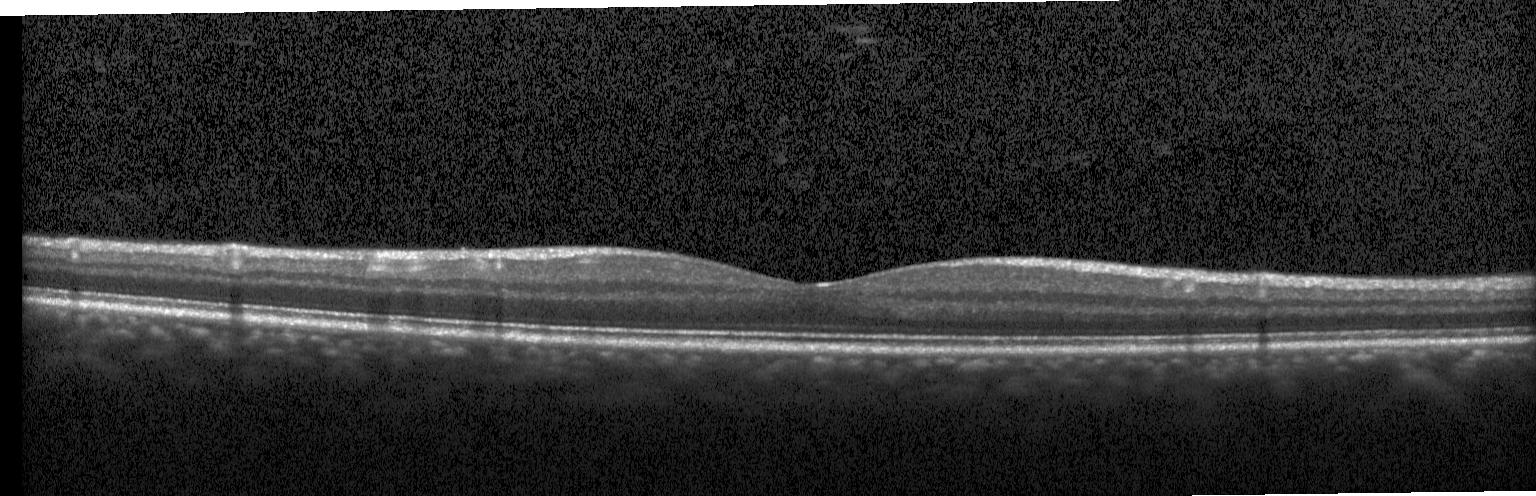

Retinal OCT B-scan. Heidelberg Spectralis OCT system. Fovea-centered
The scan shows no choroidal neovascularization, no diabetic macular edema, and no drusen.